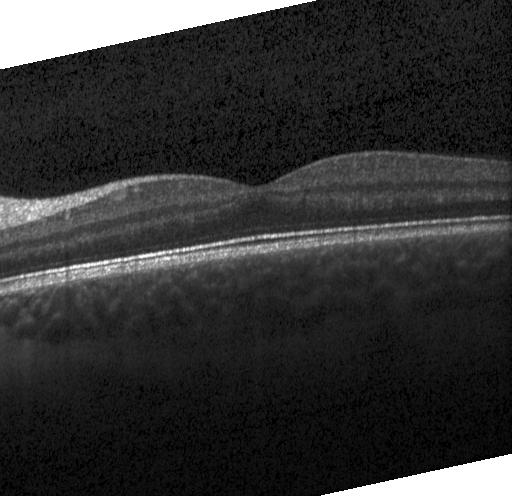
Heidelberg Spectralis OCT system. Retinal OCT cross-section
Finding: neither CNV, DME, nor drusen.